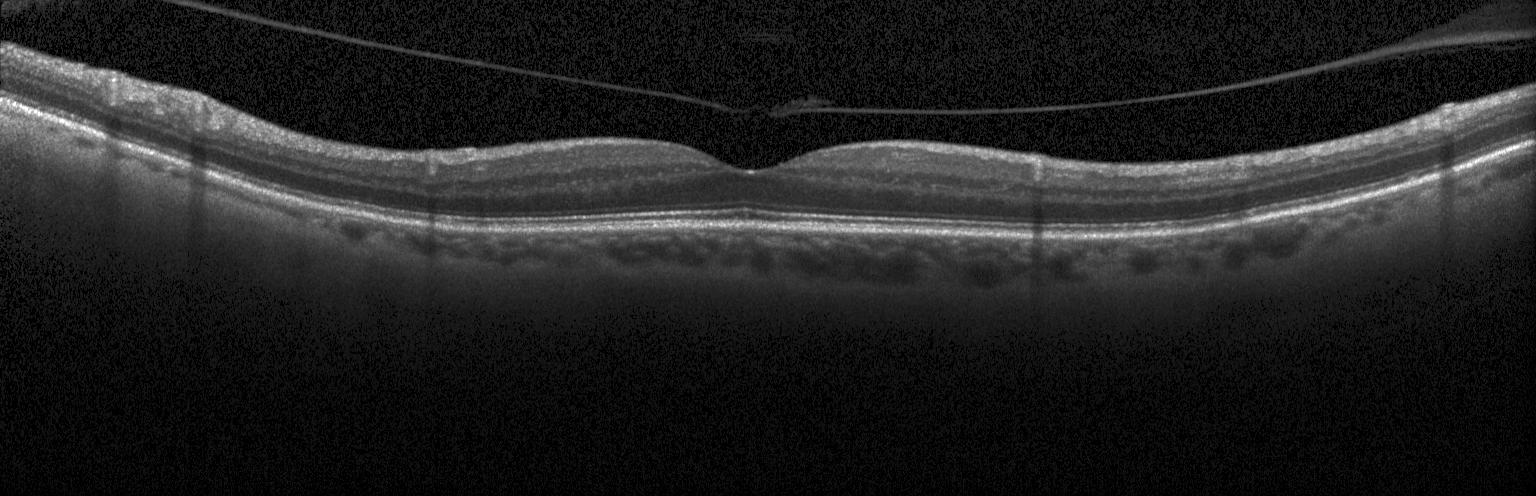 Dx: no evidence of choroidal neovascularization, diabetic macular edema, or drusen.